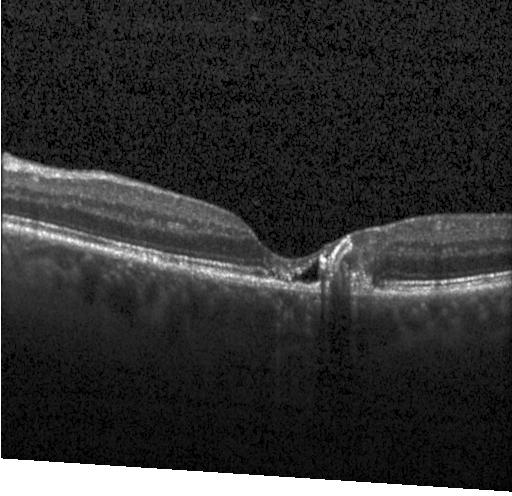 Instrument: Heidelberg Spectralis; optical coherence tomography B-scan; fovea-centered
Diagnosis: CNV.